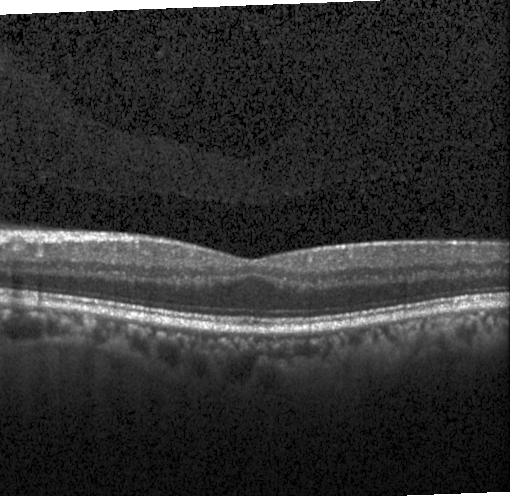

SD-OCT. OCT line scan. Diagnosis: neither CNV, DME, nor drusen.